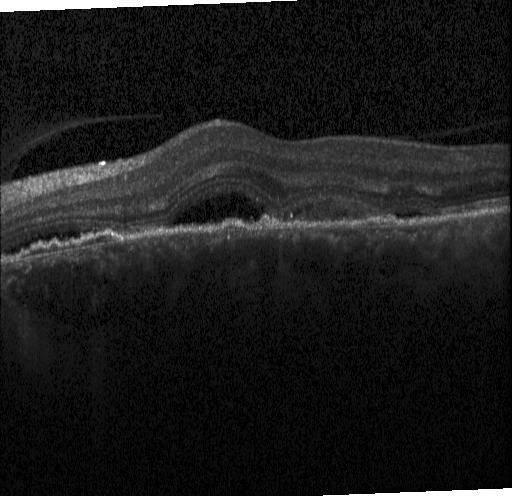
Dx: a choroidal neovascular membrane.